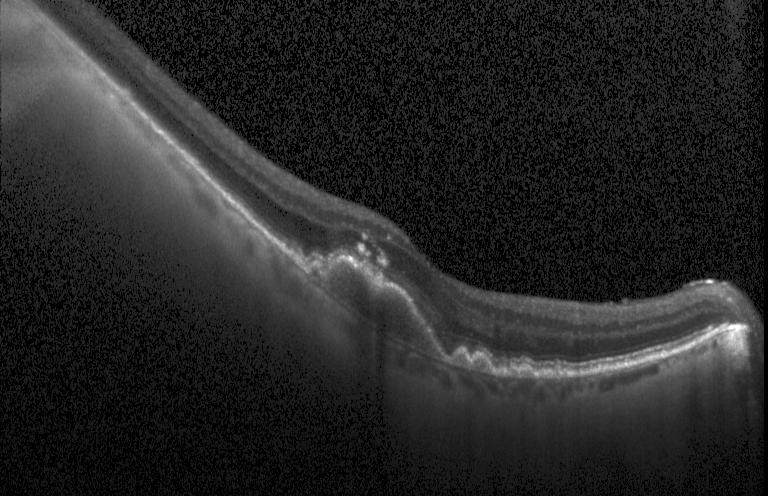

Spectral-domain OCT · retinal OCT cross-section · centered on the fovea. OCT finding: choroidal neovascularization.